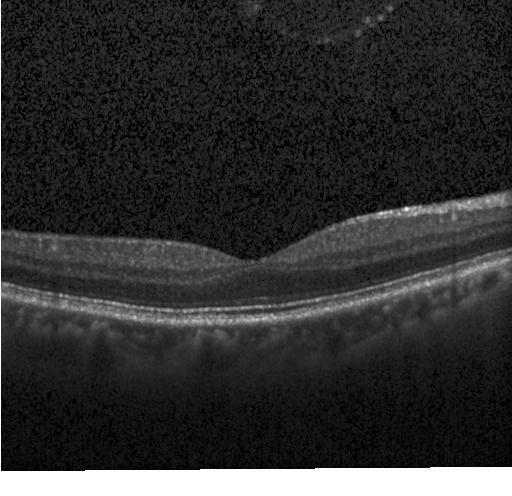

Spectral-domain OCT. Optical coherence tomography scan
Assessment: no evidence of CNV, DME, or drusen.